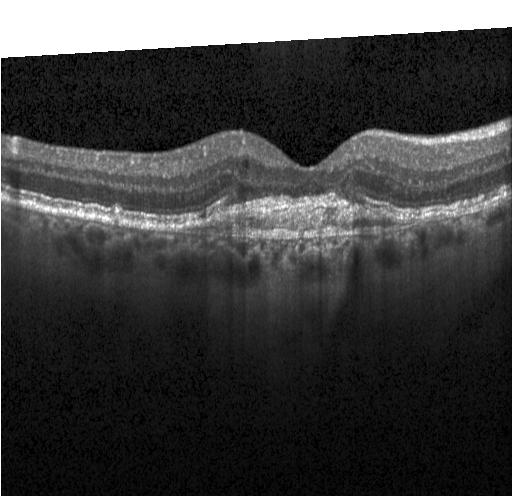 Optical coherence tomography scan. OCT finding: CNV.